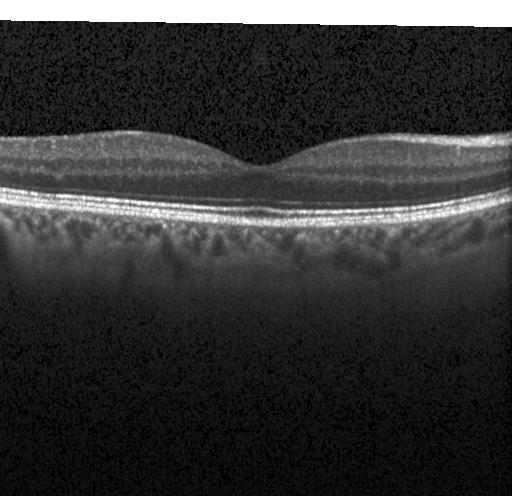

Finding: no choroidal neovascularization, diabetic macular edema, or drusen.